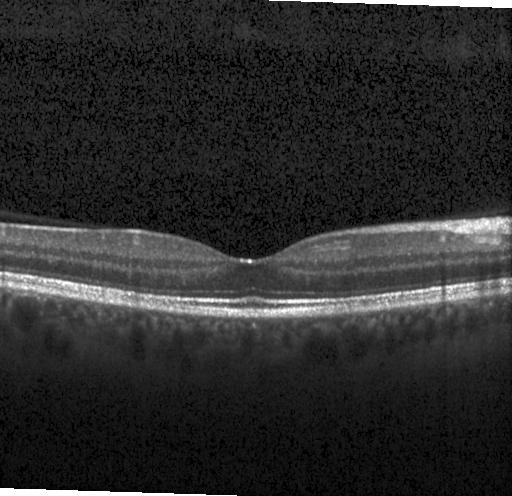
OCT B-scan
Dx: no choroidal neovascularization, diabetic macular edema, or drusen.